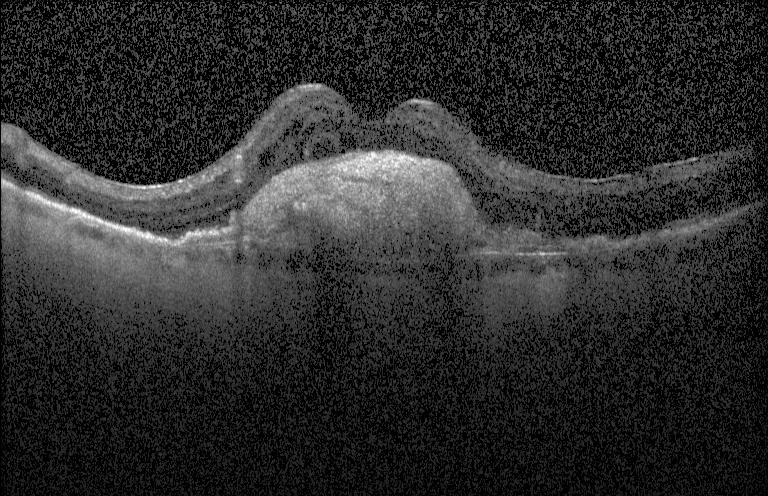 Finding: choroidal neovascularization.